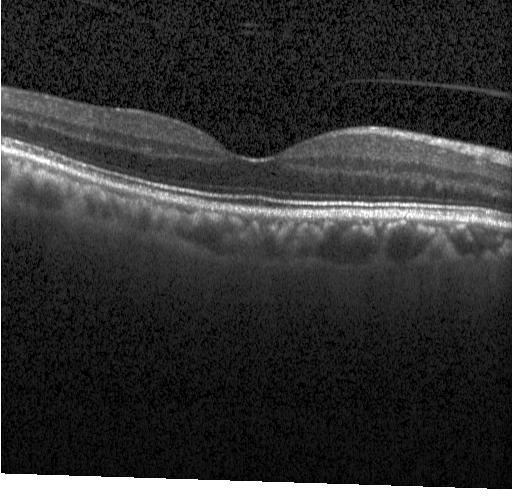 Acquired on a Heidelberg Spectralis; optical coherence tomography scan; centered on the fovea; SD-OCT.
Diagnosis: no evidence of choroidal neovascularization, diabetic macular edema, or drusen.